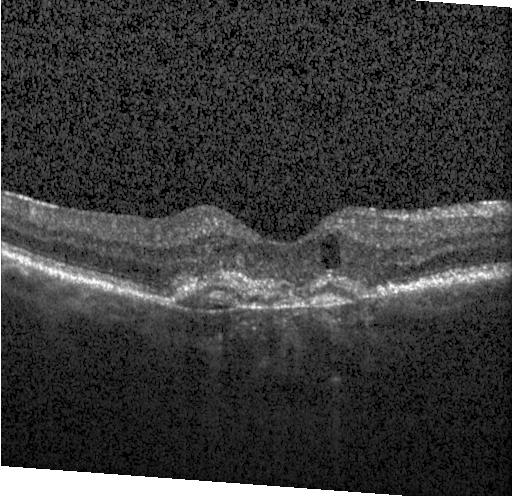
Fovea-centered, spectral-domain OCT, OCT line scan
Dx: choroidal neovascularization (CNV).